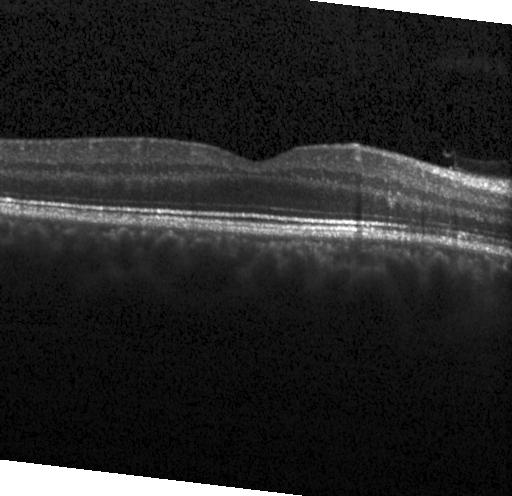

No choroidal neovascularization, diabetic macular edema, or drusen.